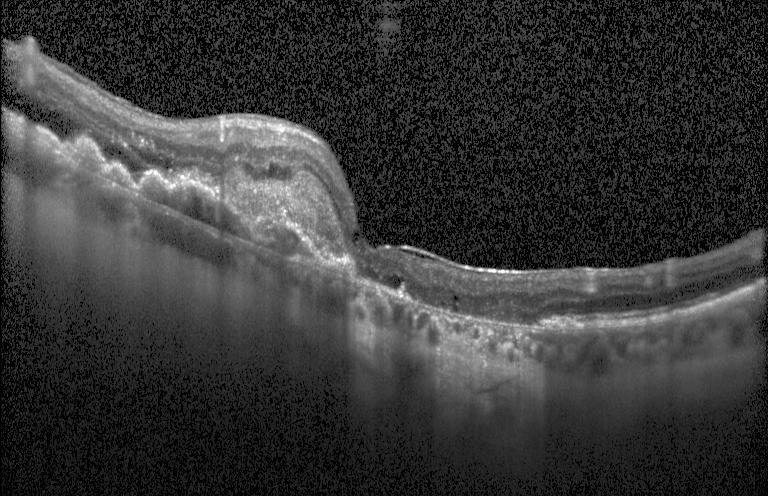 Instrument: Heidelberg Spectralis; OCT line scan; SD-OCT. This B-scan demonstrates a choroidal neovascular membrane.